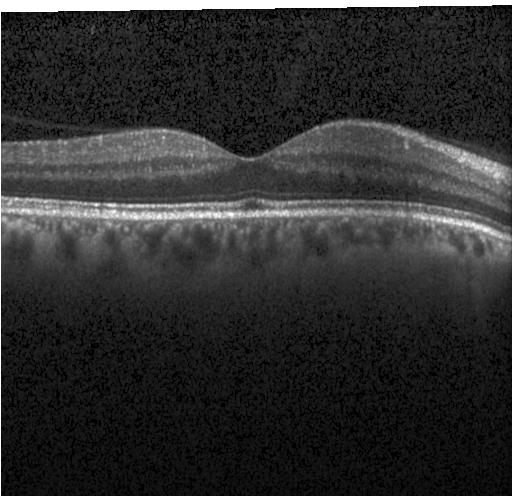 Optical coherence tomography B-scan. Acquired on a Heidelberg Spectralis. Spectral-domain optical coherence tomography
The scan shows neither choroidal neovascularization, diabetic macular edema, nor drusen.